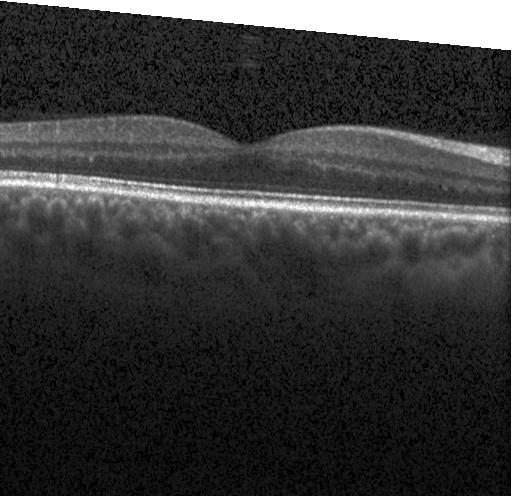

OCT line scan. Dx: no choroidal neovascularization, diabetic macular edema, or drusen.